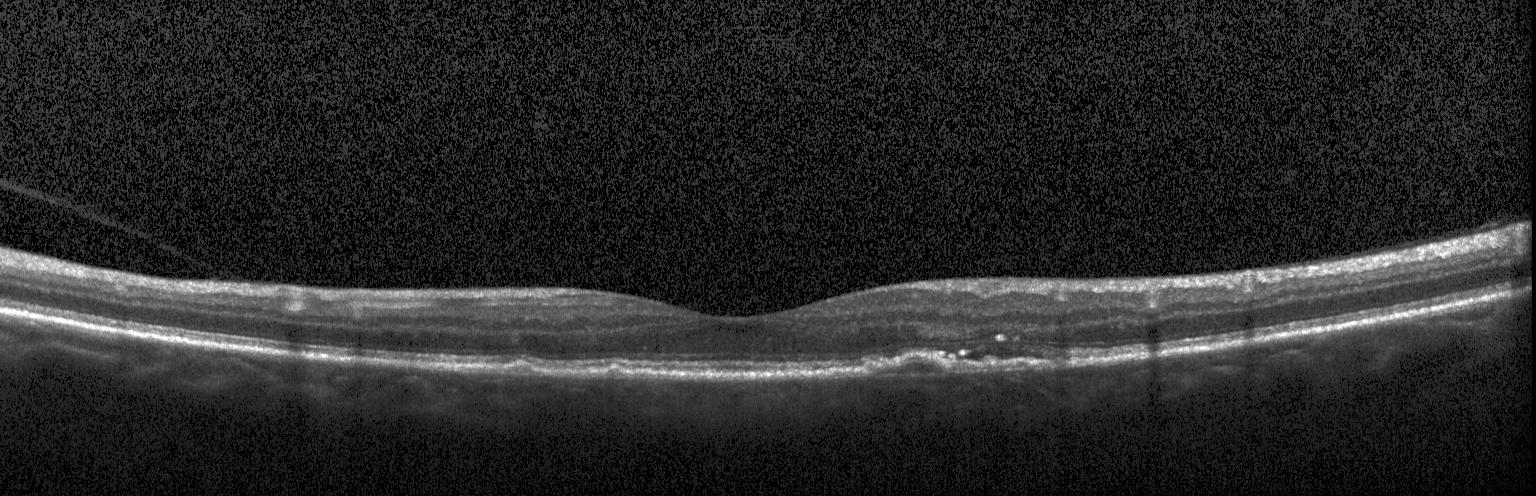

OCT B-scan.
OCT finding: choroidal neovascularization (CNV).